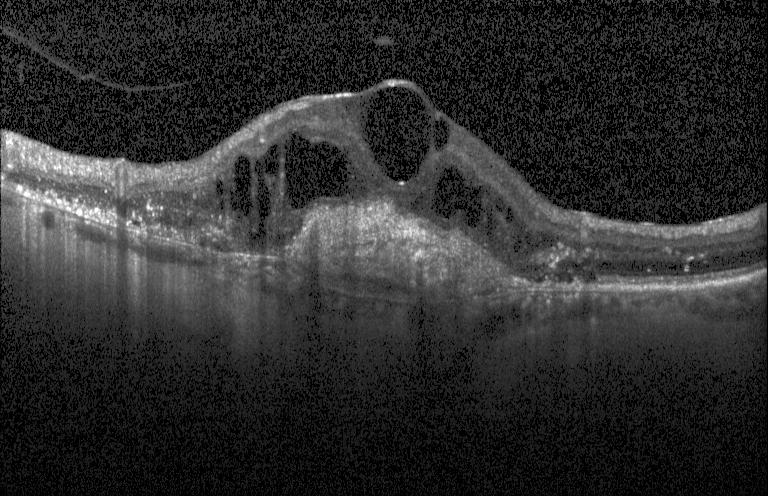 OCT finding: a choroidal neovascular membrane.